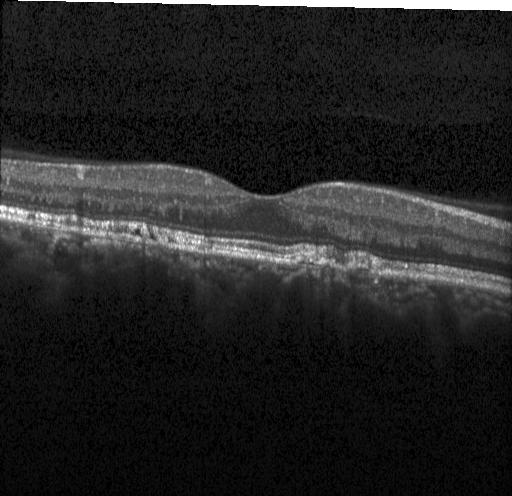
Centered on the fovea. Optical coherence tomography scan. Impression: drusen.